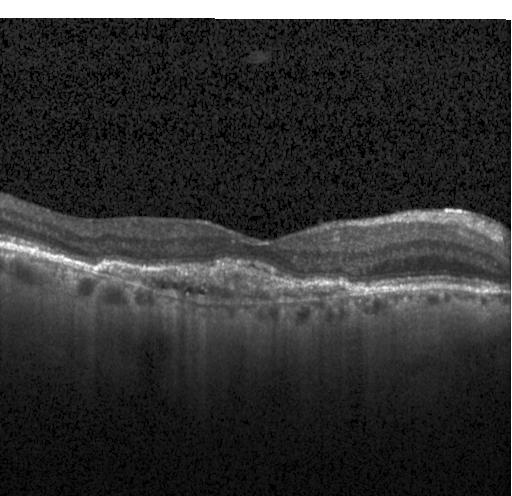

Spectral-domain optical coherence tomography · acquired on a Heidelberg Spectralis · centered on the fovea · retinal OCT B-scan. The scan shows choroidal neovascularization (CNV).